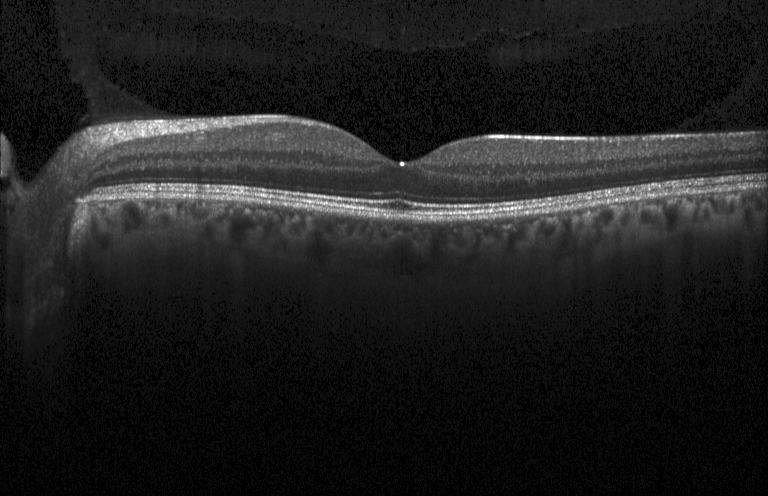 Retinal OCT cross-section. Horizontal scan through the fovea
Finding: no choroidal neovascularization, diabetic macular edema, or drusen.